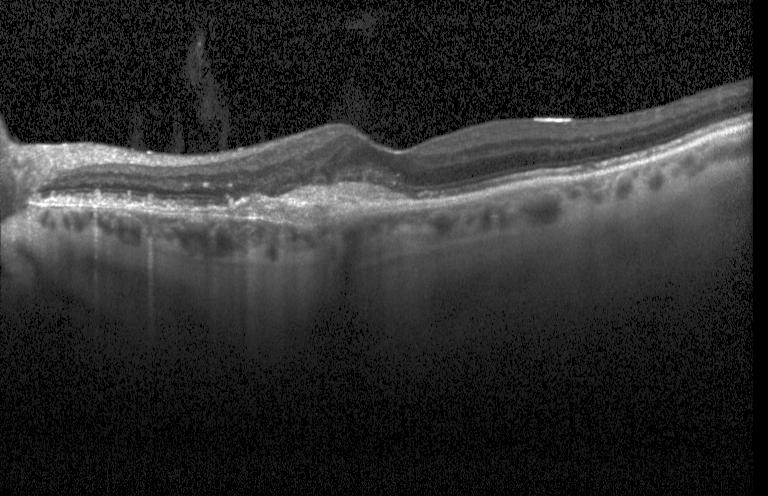
Finding: choroidal neovascularization (CNV).